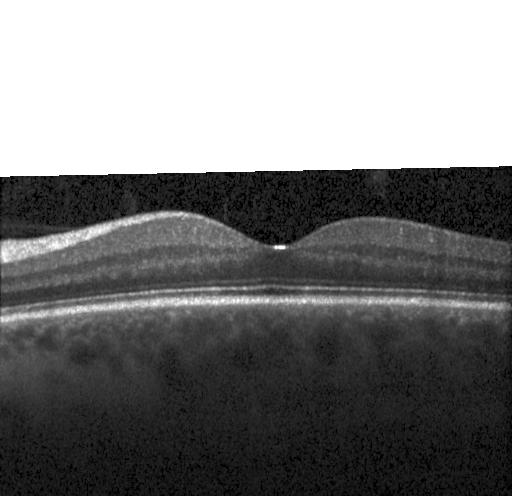

No choroidal neovascularization, diabetic macular edema, or drusen.